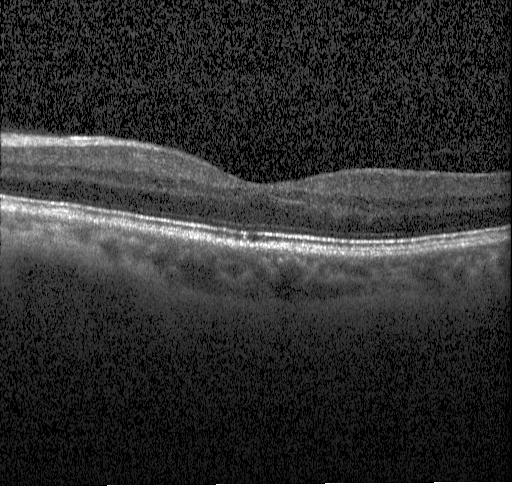 Centered on the fovea · retinal OCT cross-section · Heidelberg Spectralis · spectral-domain OCT. Assessment: neither CNV, DME, nor drusen.